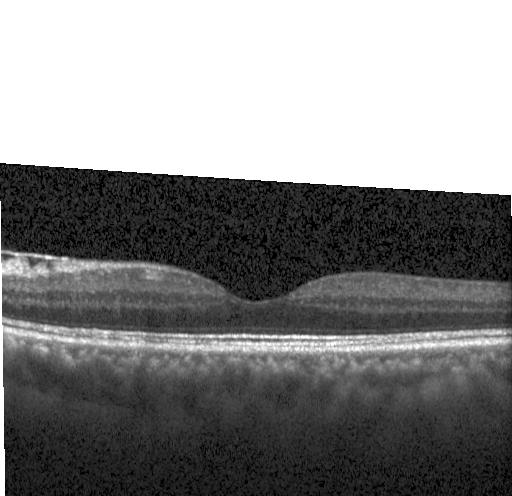

Macular OCT: no choroidal neovascularization, diabetic macular edema, or drusen.